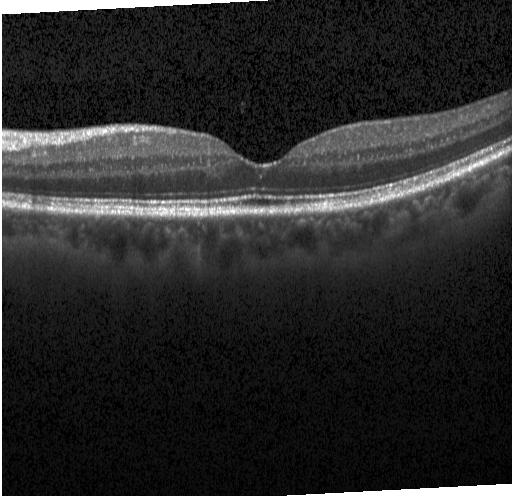

Diagnosis: no CNV, DME, or drusen.